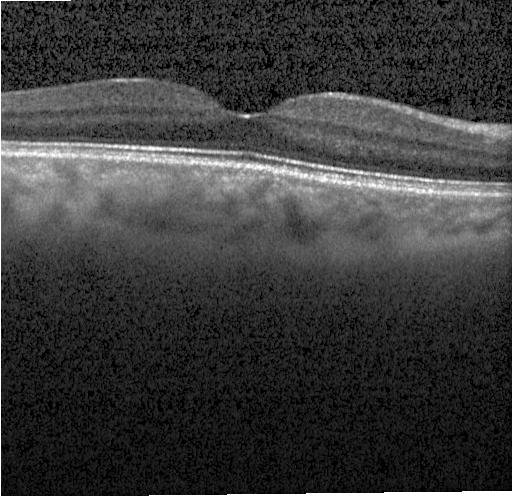

Macular OCT demonstrating no evidence of CNV, DME, or drusen.